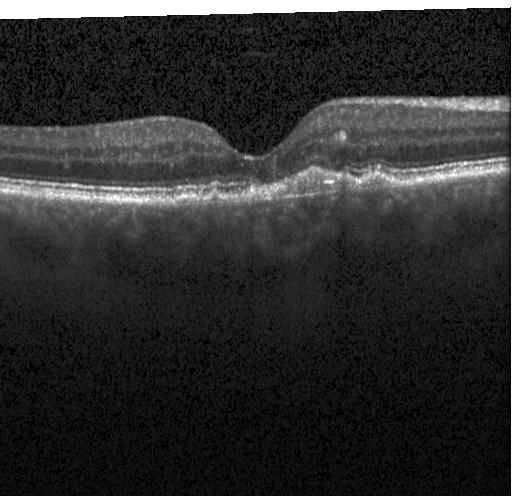 Retinal OCT B-scan
Dx: choroidal neovascularization (CNV).